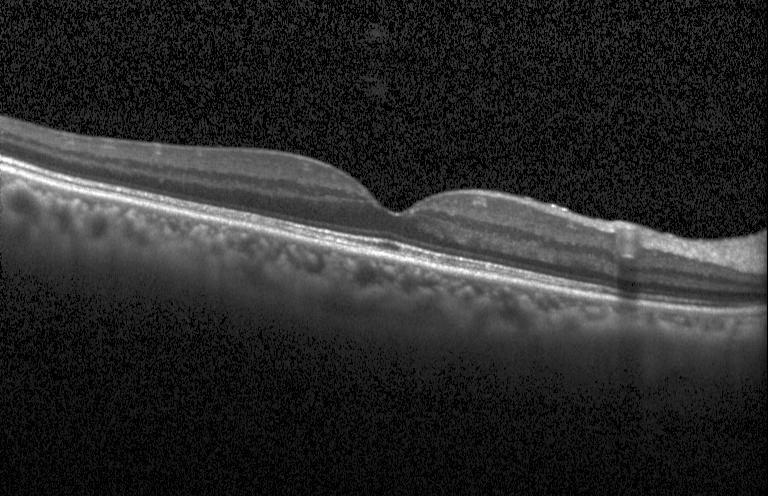
Finding: neither choroidal neovascularization, diabetic macular edema, nor drusen.